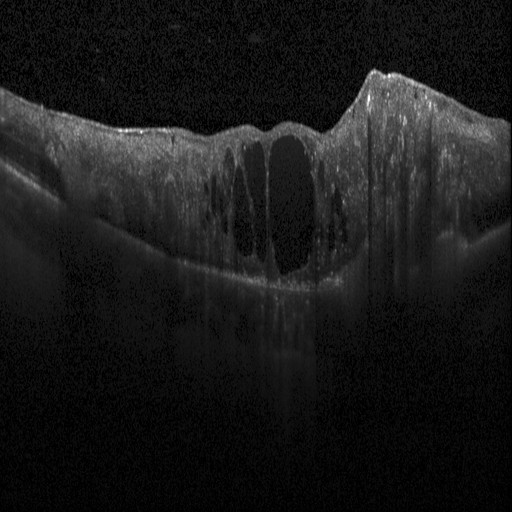
Through the macula. Spectral-domain optical coherence tomography. Optical coherence tomography B-scan. Instrument: Heidelberg Spectralis — Diagnosis: diabetic macular edema.